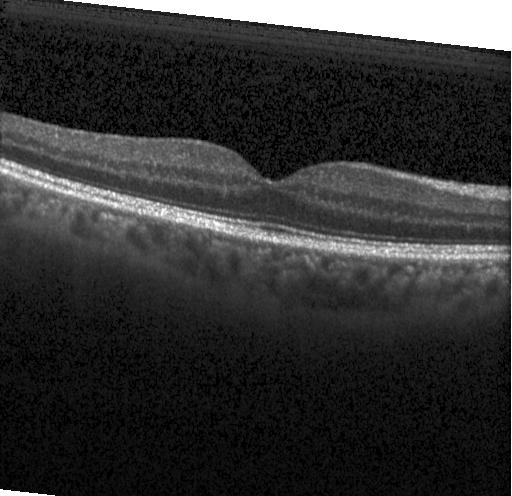

Macular OCT: no evidence of CNV, DME, or drusen.